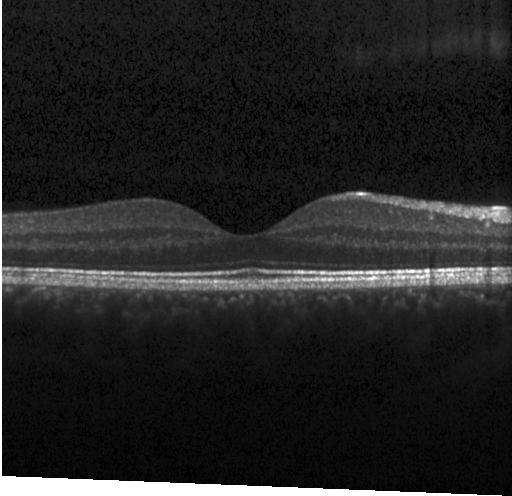 OCT B-scan showing no choroidal neovascularization, no diabetic macular edema, and no drusen.